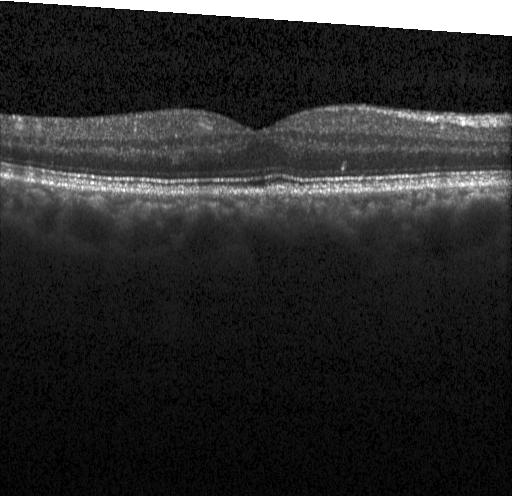
Impression: no choroidal neovascularization, no diabetic macular edema, and no drusen.